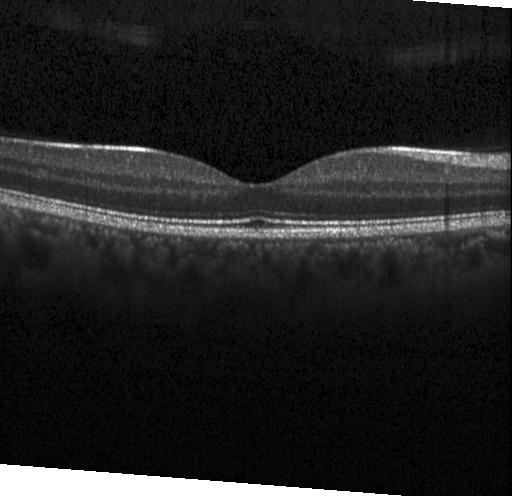
Optical coherence tomography B-scan.
Impression: no evidence of choroidal neovascularization, diabetic macular edema, or drusen.